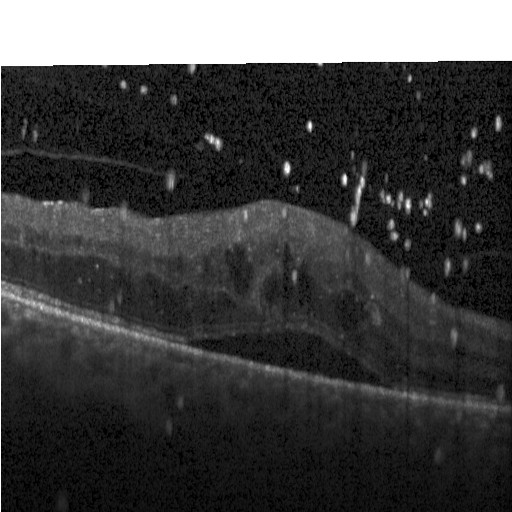
This B-scan demonstrates diabetic macular edema (DME).